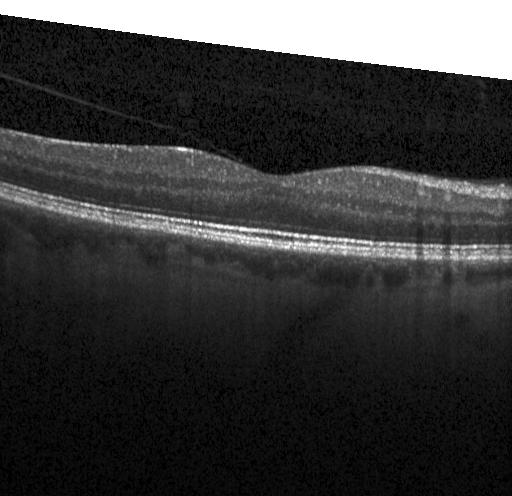

SD-OCT. Optical coherence tomography scan. Centered on the fovea. Acquired on a Heidelberg Spectralis. Macular OCT: no CNV, DME, or drusen.